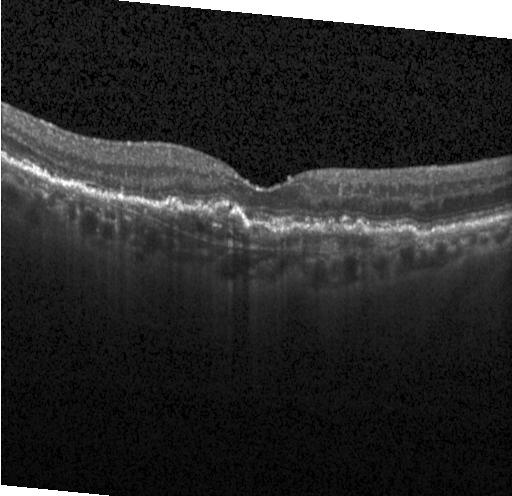

OCT B-scan showing choroidal neovascularization.